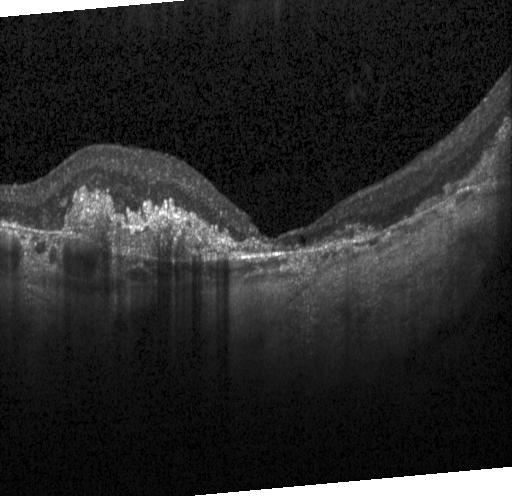
Diagnosis: choroidal neovascularization (CNV).